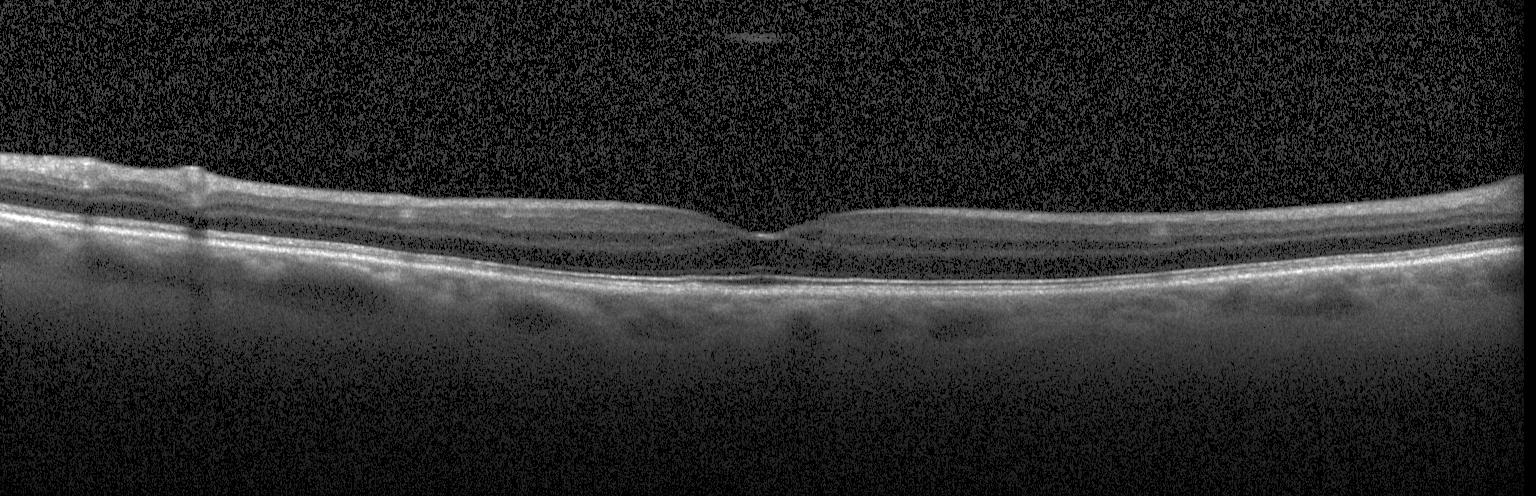

No CNV, no DME, and no drusen.